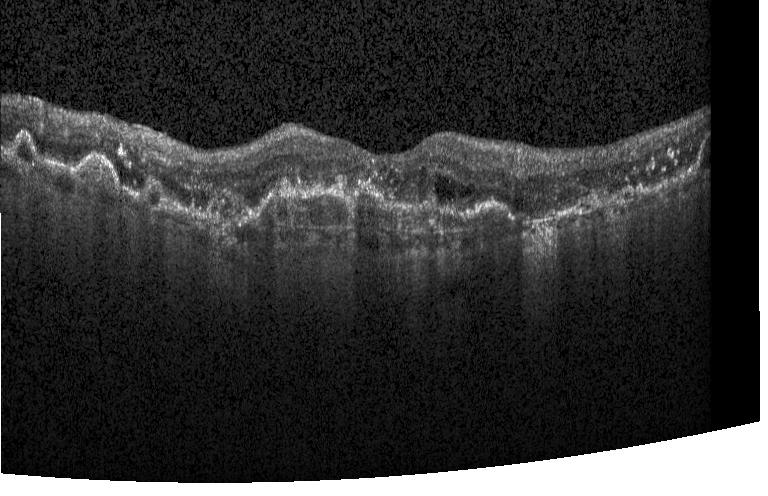 Optical coherence tomography B-scan — OCT finding: a choroidal neovascular membrane.